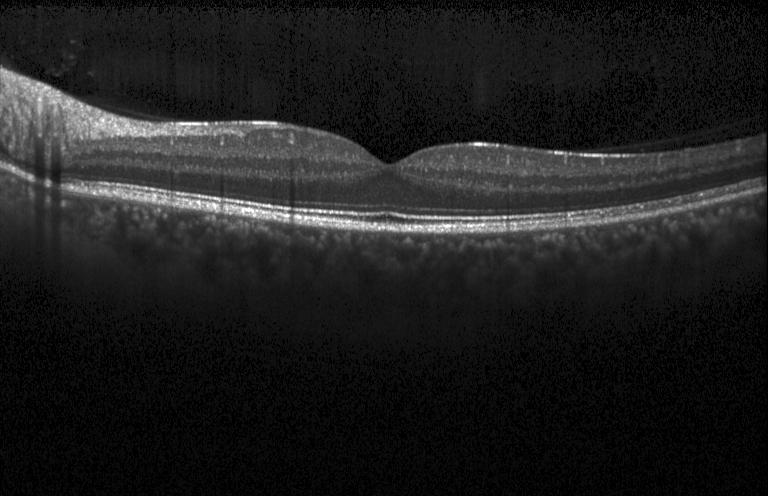 Optical coherence tomography scan — Assessment: no CNV, DME, or drusen.